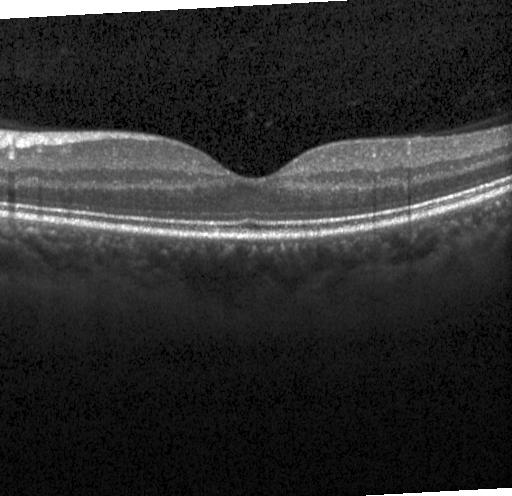

Heidelberg Spectralis · through the macula · OCT B-scan.
Assessment: no evidence of choroidal neovascularization, diabetic macular edema, or drusen.